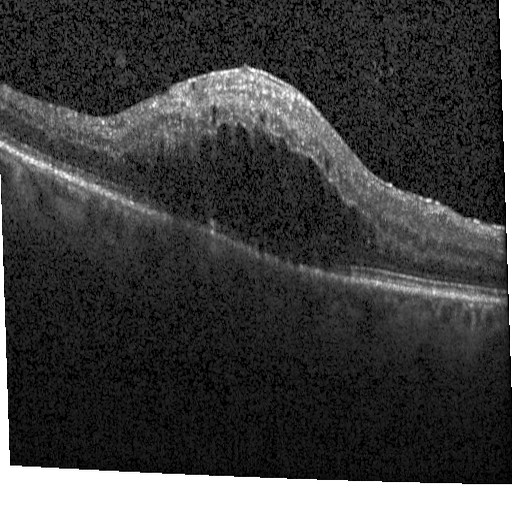 Spectral-domain optical coherence tomography, macular scan, OCT B-scan
Diagnosis: DME.